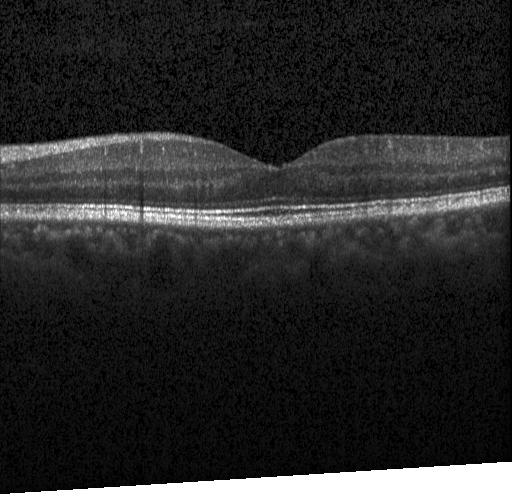
Through the macula, optical coherence tomography scan — Finding: neither choroidal neovascularization, diabetic macular edema, nor drusen.